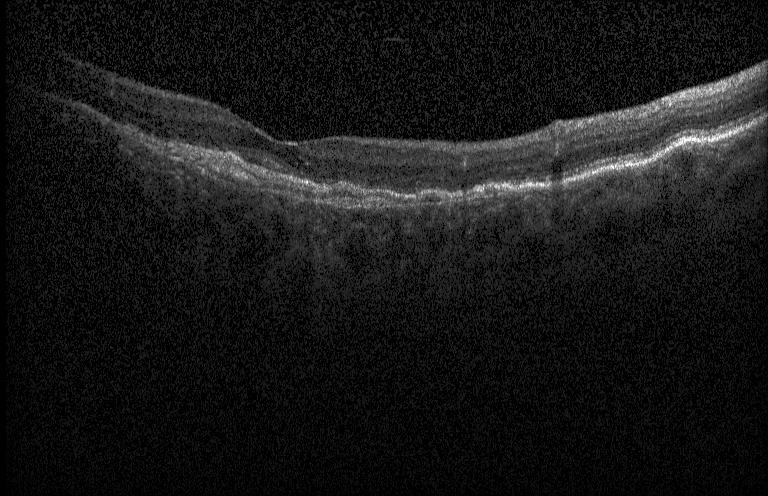

A choroidal neovascular membrane.